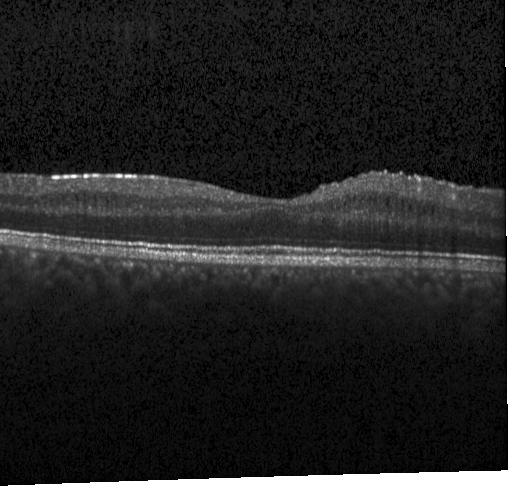
OCT B-scan, instrument: Heidelberg Spectralis
Impression: DME.